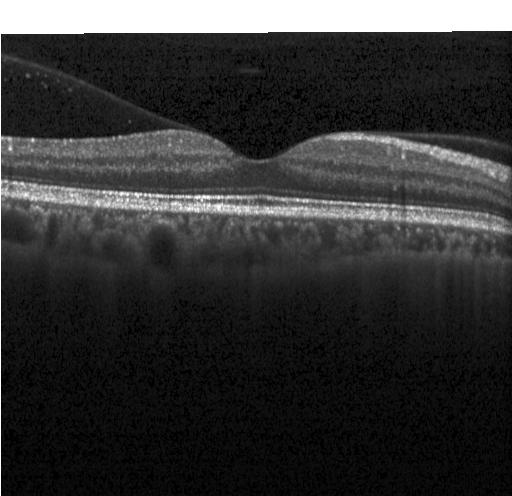

OCT B-scan
Finding: no choroidal neovascularization, no diabetic macular edema, and no drusen.